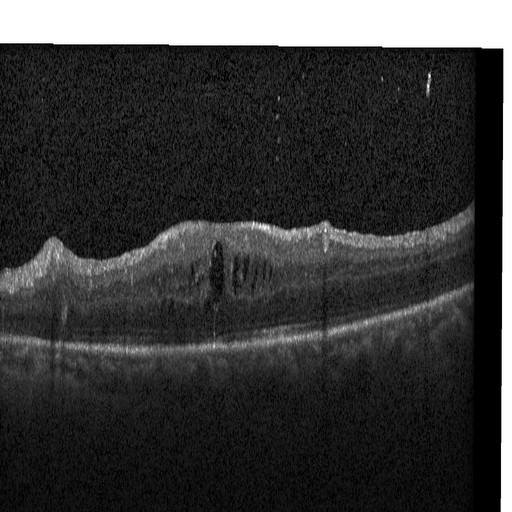
OCT B-scan — Macular OCT: diabetic macular edema (DME).